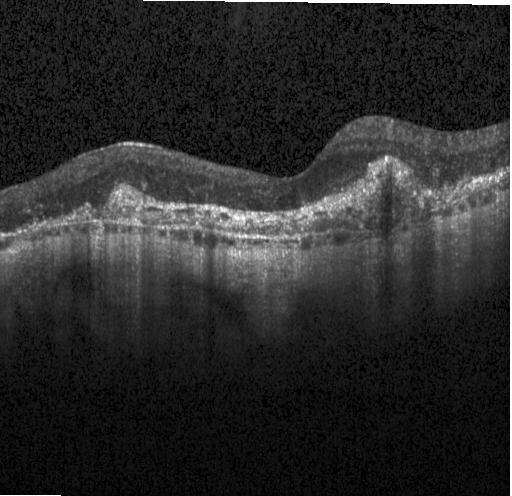 Macular scan, OCT line scan, Heidelberg Spectralis OCT system, SD-OCT
Impression: choroidal neovascularization.